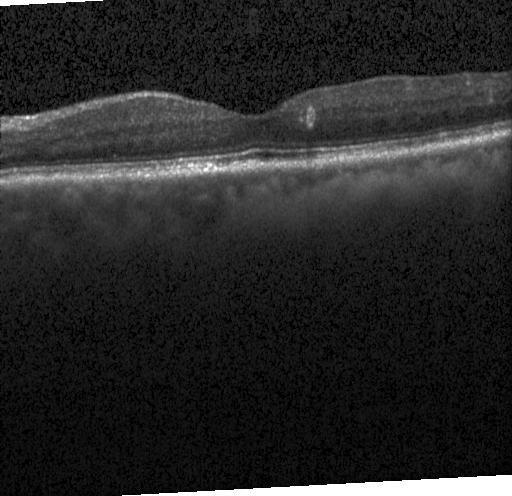

OCT B-scan. Impression: no choroidal neovascularization, no diabetic macular edema, and no drusen.